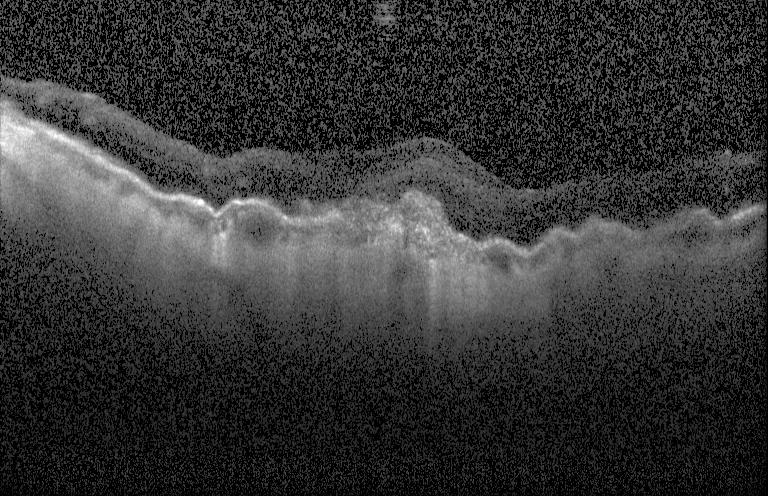

Finding: CNV.